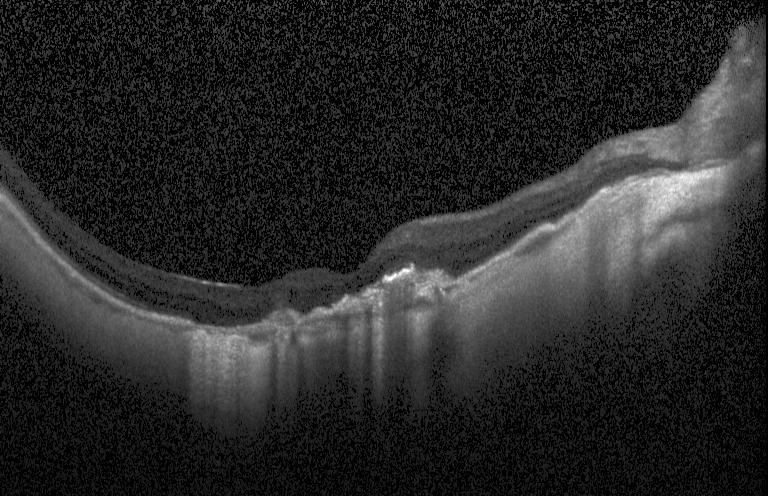 Retinal OCT B-scan. SD-OCT. Heidelberg Spectralis OCT system. Through the macula — Impression: choroidal neovascularization (CNV).